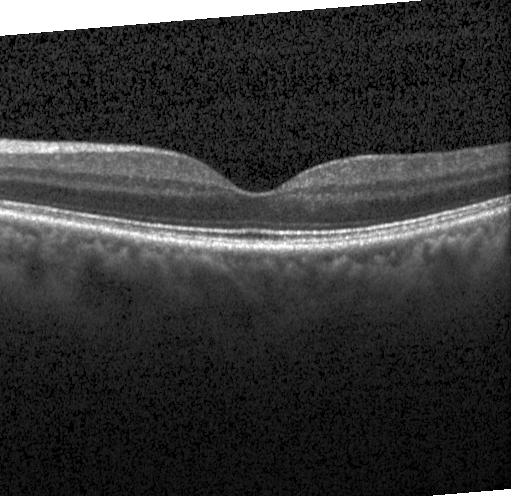

Dx: no choroidal neovascularization, no diabetic macular edema, and no drusen.